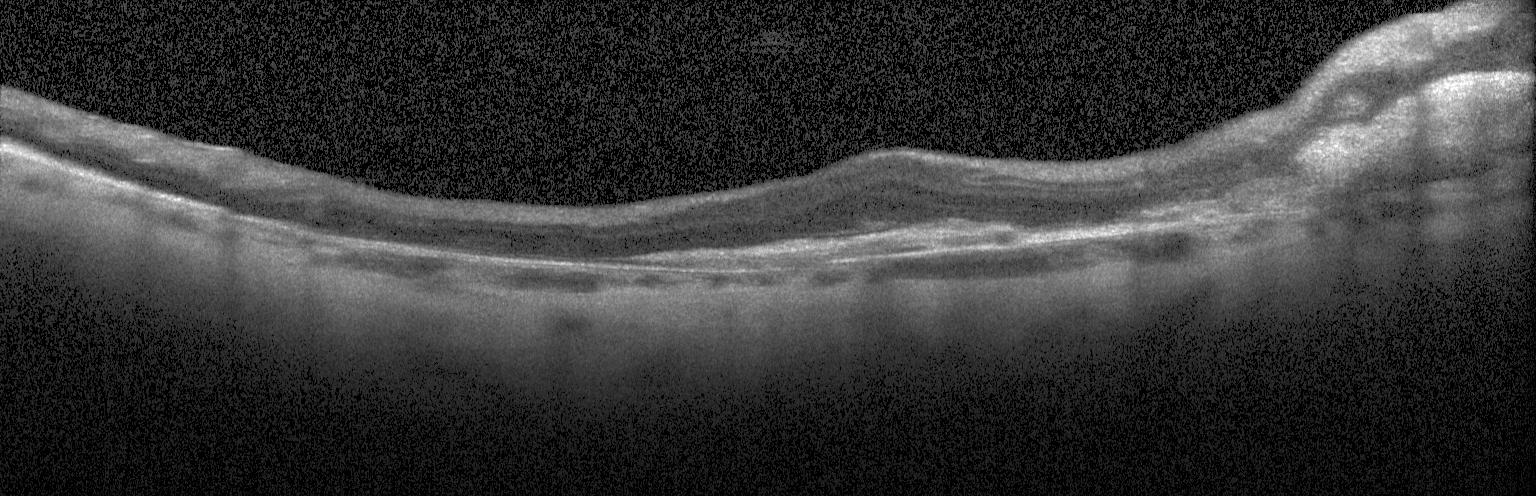
Diagnosis: CNV.